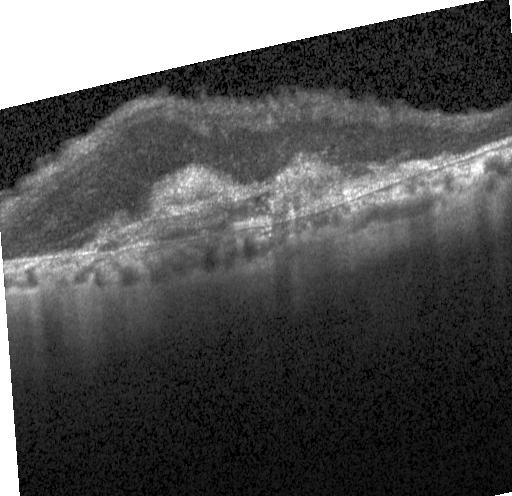 OCT B-scan. Diagnosis: a choroidal neovascular membrane.